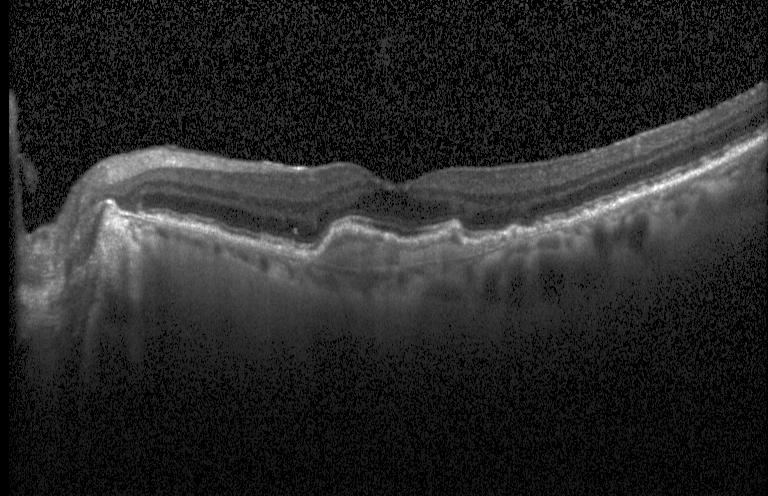

Optical coherence tomography scan. Impression: a choroidal neovascular membrane.